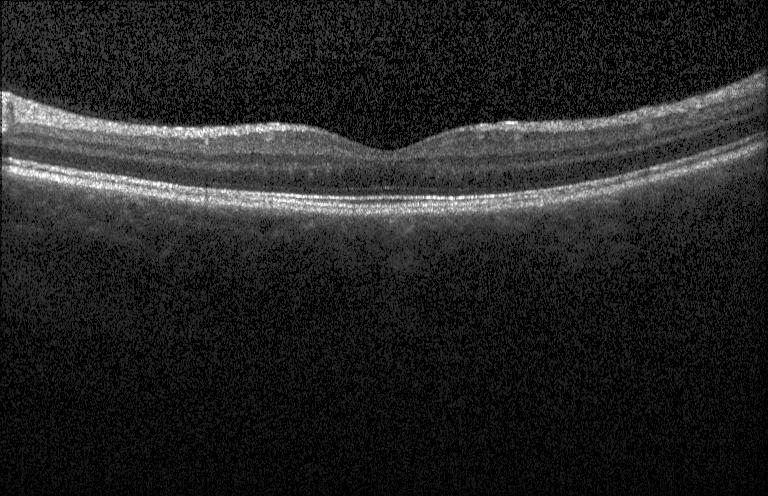

OCT scan showing neither CNV, DME, nor drusen.